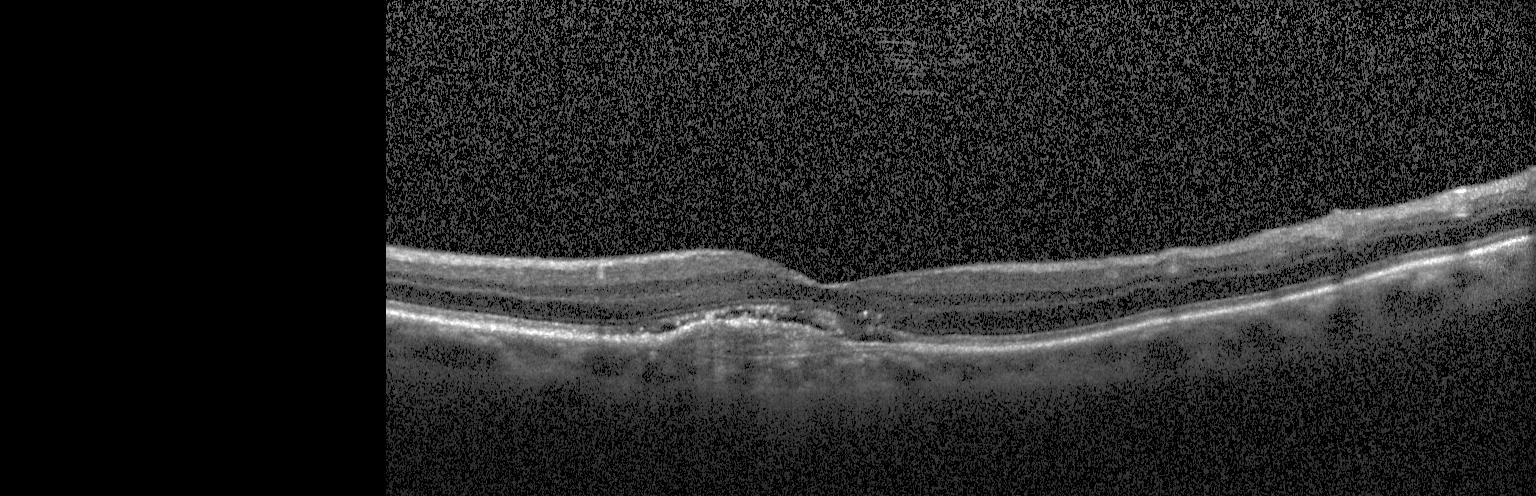

Heidelberg Spectralis OCT system, SD-OCT, OCT line scan — Macular OCT: CNV.